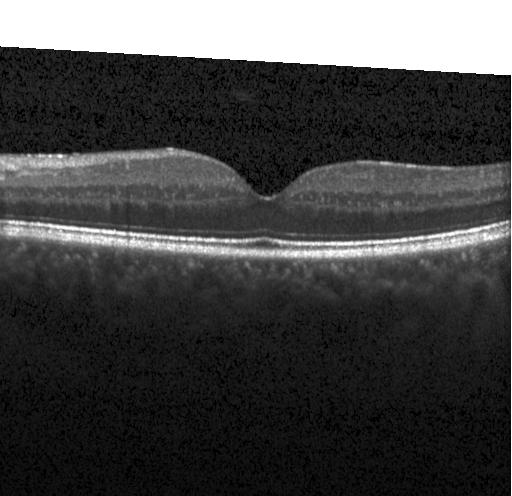 Impression: no choroidal neovascularization, no diabetic macular edema, and no drusen.